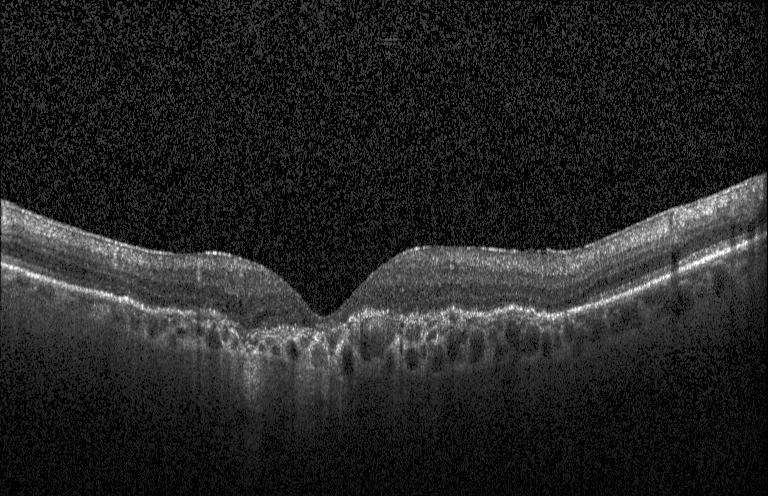

Finding: a choroidal neovascular membrane.